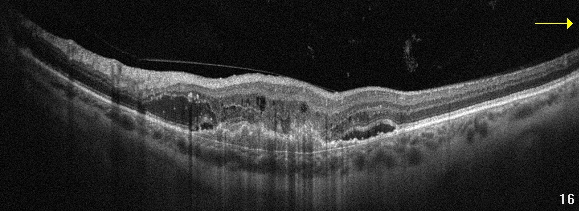 OCT B-scan showing age-related macular degeneration (AMD).